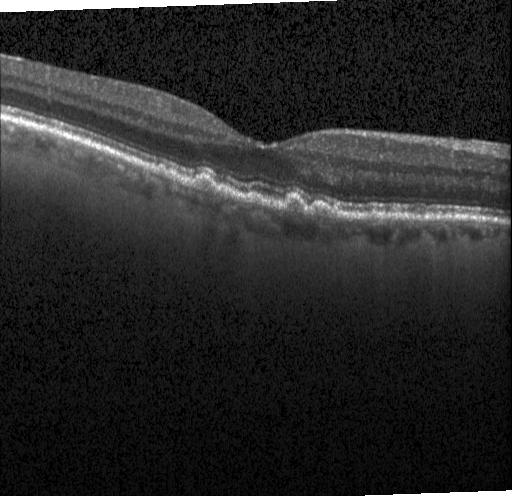
Instrument: Heidelberg Spectralis; optical coherence tomography B-scan; spectral-domain optical coherence tomography; fovea-centered. Dx: sub-RPE drusenoid deposits.